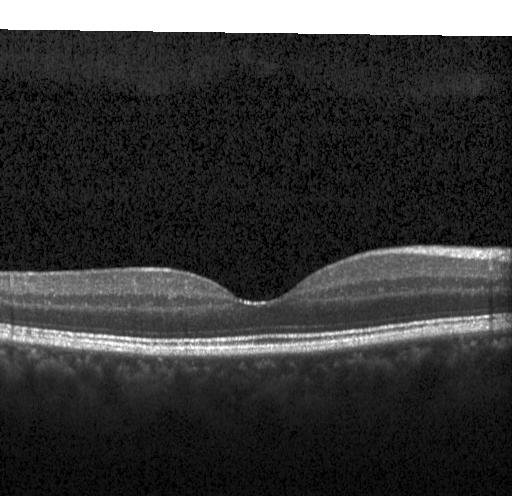
Spectral-domain OCT, centered on the fovea, OCT line scan
Impression: no choroidal neovascularization, diabetic macular edema, or drusen.